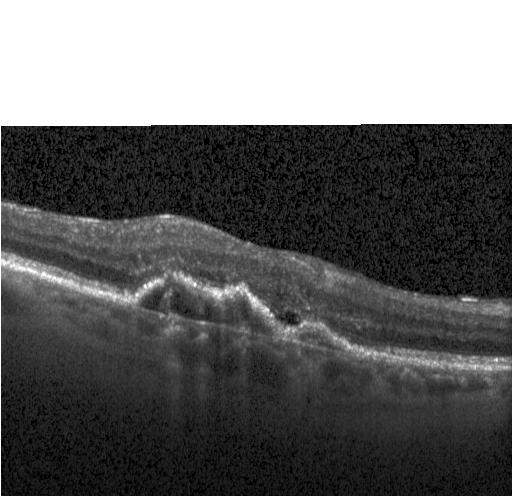 Spectral-domain OCT B-scan: choroidal neovascularization.